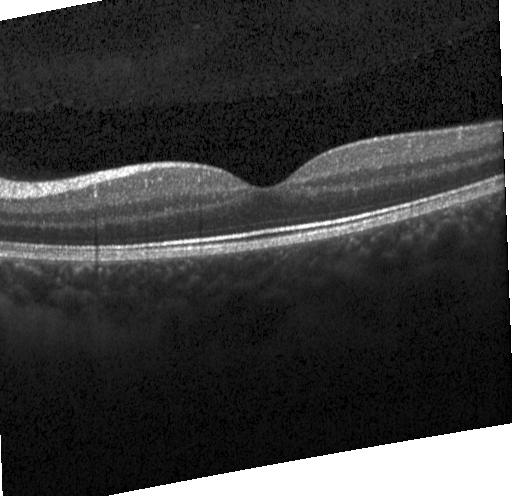
Retinal OCT cross-section — Impression: no evidence of choroidal neovascularization, diabetic macular edema, or drusen.